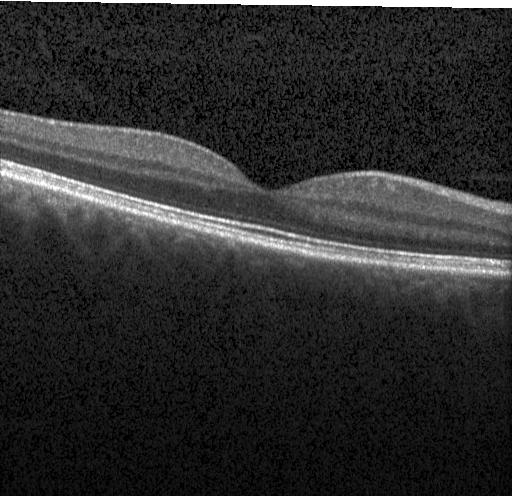 Optical coherence tomography B-scan.
No choroidal neovascularization, diabetic macular edema, or drusen.